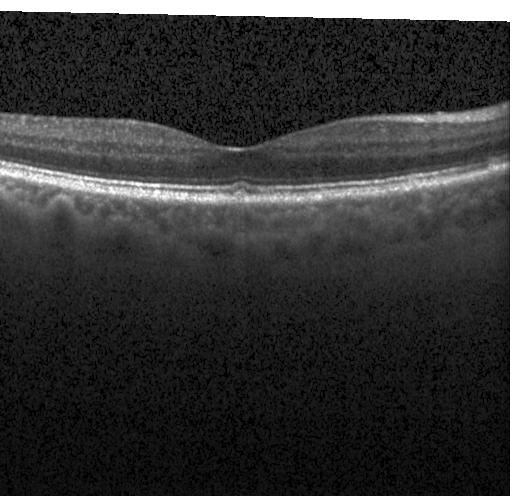
Diagnosis: no evidence of choroidal neovascularization, diabetic macular edema, or drusen.